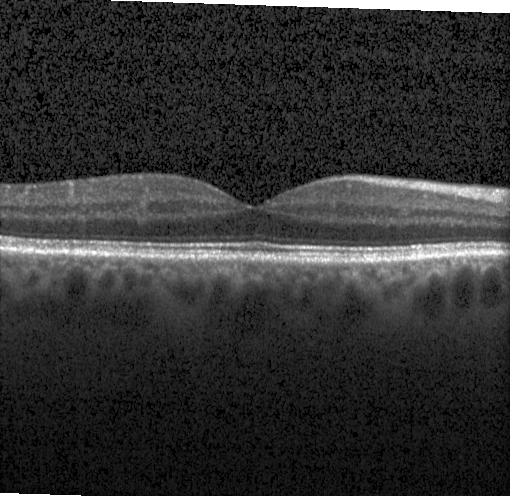
Finding: no choroidal neovascularization, diabetic macular edema, or drusen.